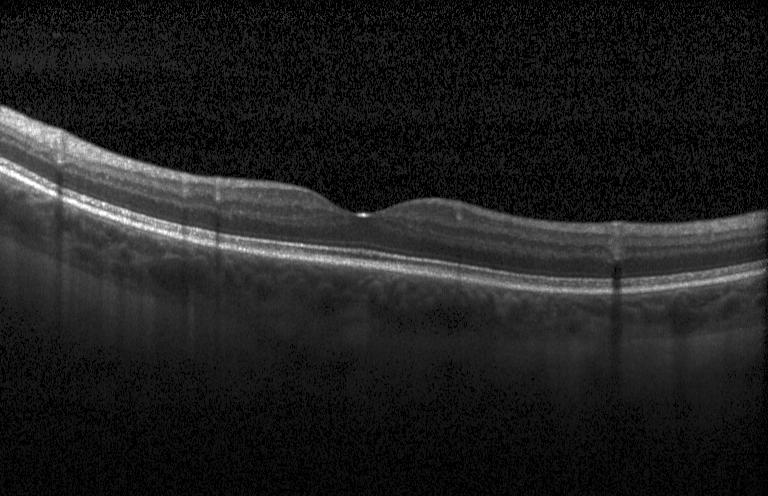 Dx: no CNV, DME, or drusen.